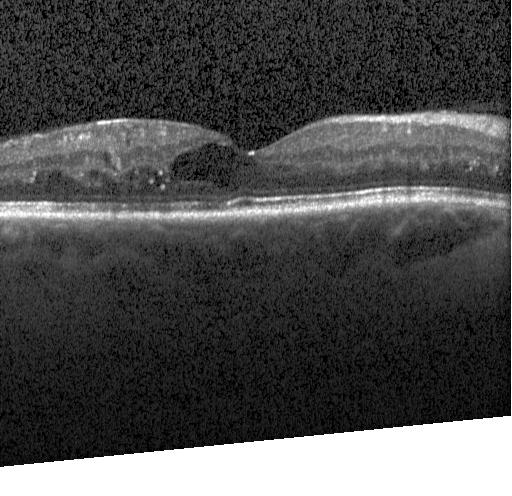

Retinal OCT cross-section. Centered on the fovea
DME.